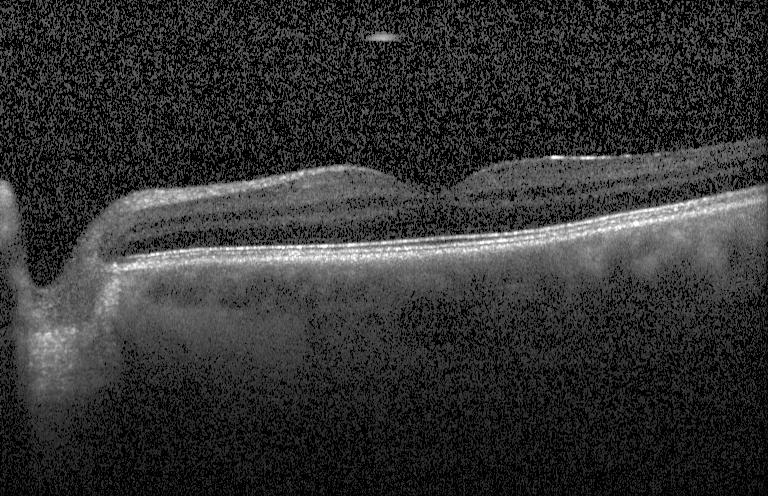 OCT B-scan.
Finding: no evidence of choroidal neovascularization, diabetic macular edema, or drusen.